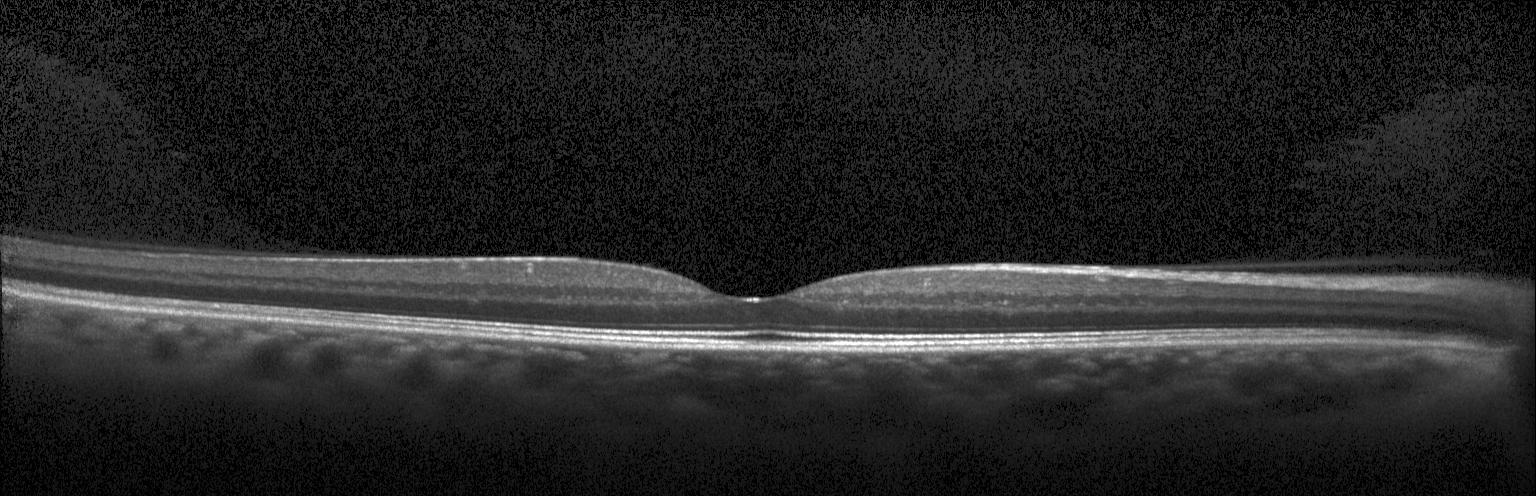

Optical coherence tomography scan, horizontal scan through the fovea, acquired on a Heidelberg Spectralis, spectral-domain optical coherence tomography
Finding: no choroidal neovascularization, diabetic macular edema, or drusen.